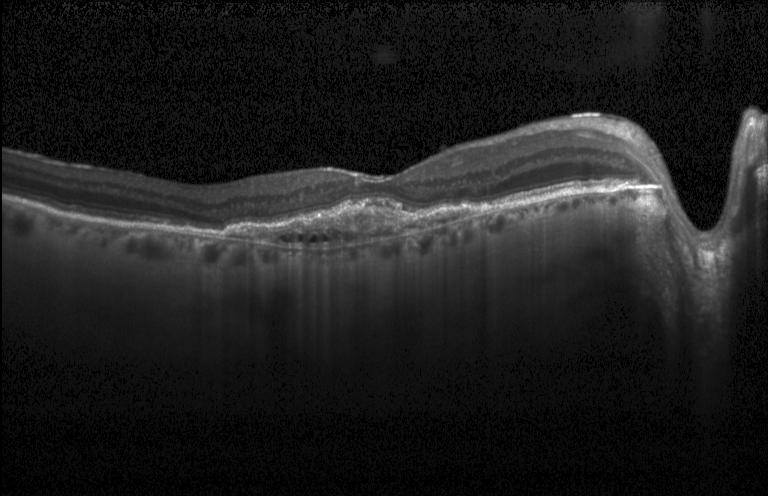
OCT line scan.
Macular OCT: choroidal neovascularization.